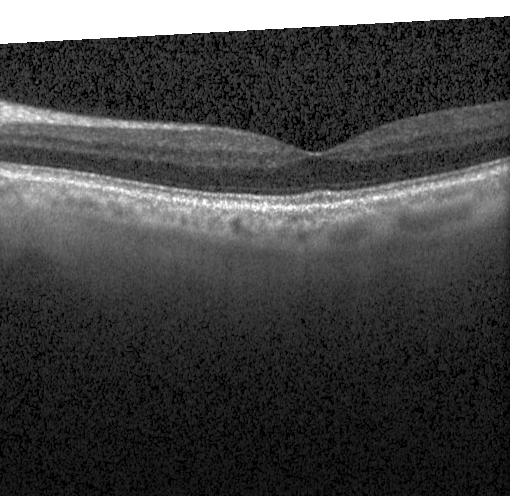 Retinal OCT cross-section — Macular OCT: no evidence of choroidal neovascularization, diabetic macular edema, or drusen.